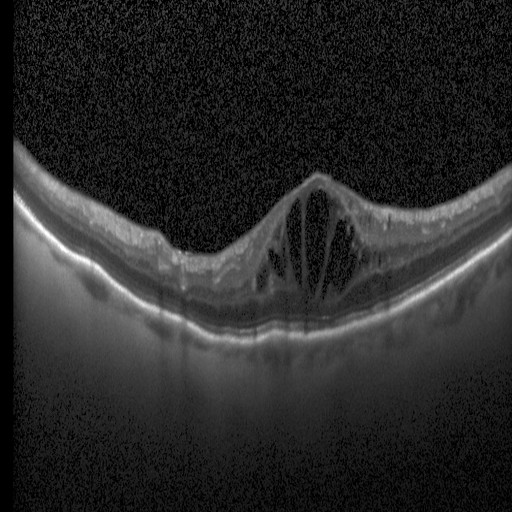

Heidelberg Spectralis, fovea-centered, OCT line scan. Diabetic macular edema.